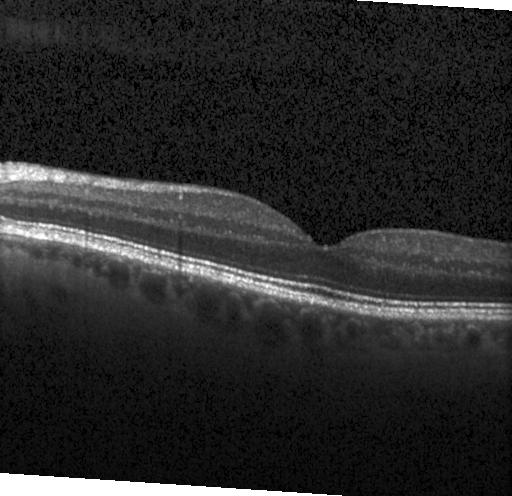 OCT B-scan
Assessment: no CNV, no DME, and no drusen.